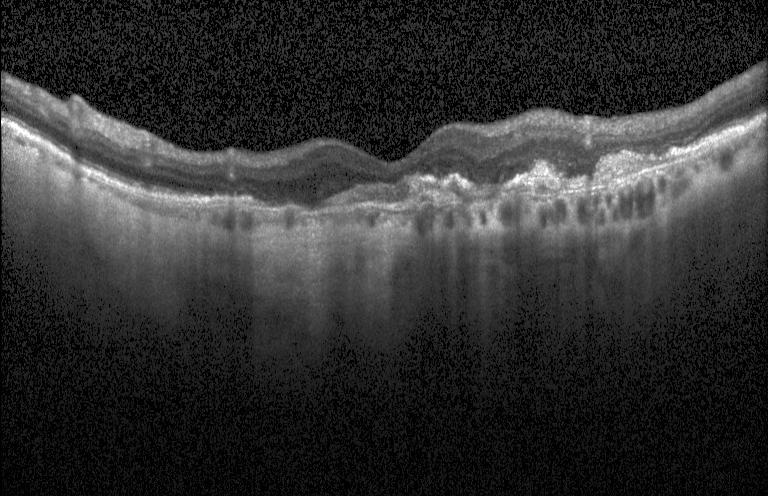 OCT B-scan. Diagnosis: CNV.